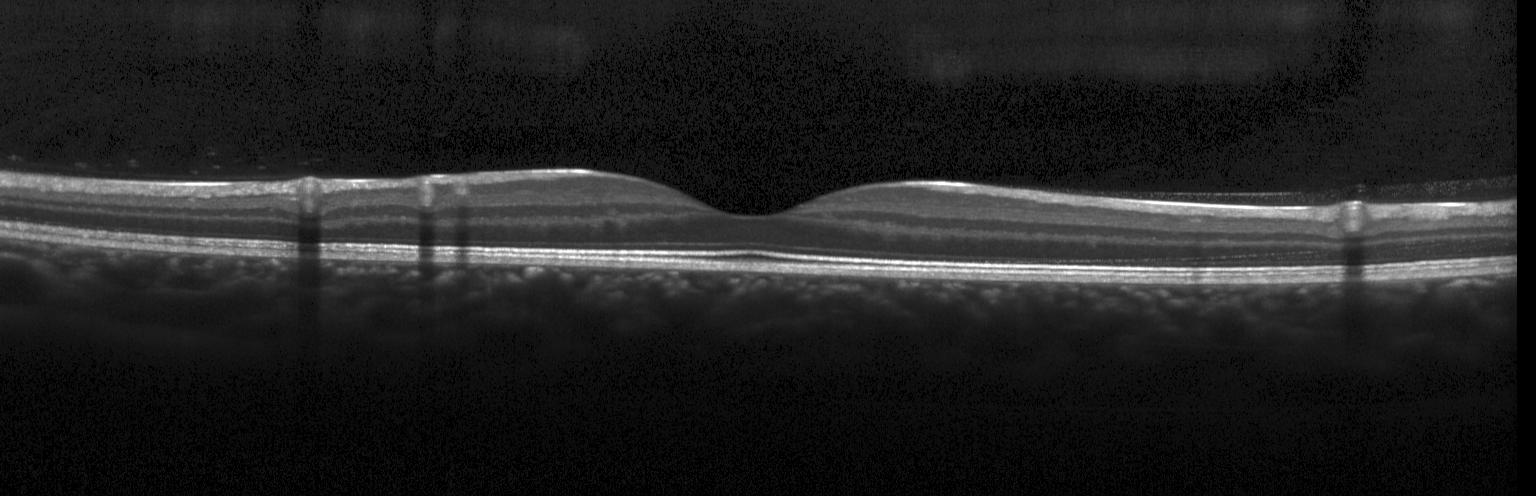 Instrument: Heidelberg Spectralis. Optical coherence tomography scan. Impression: no choroidal neovascularization, diabetic macular edema, or drusen.